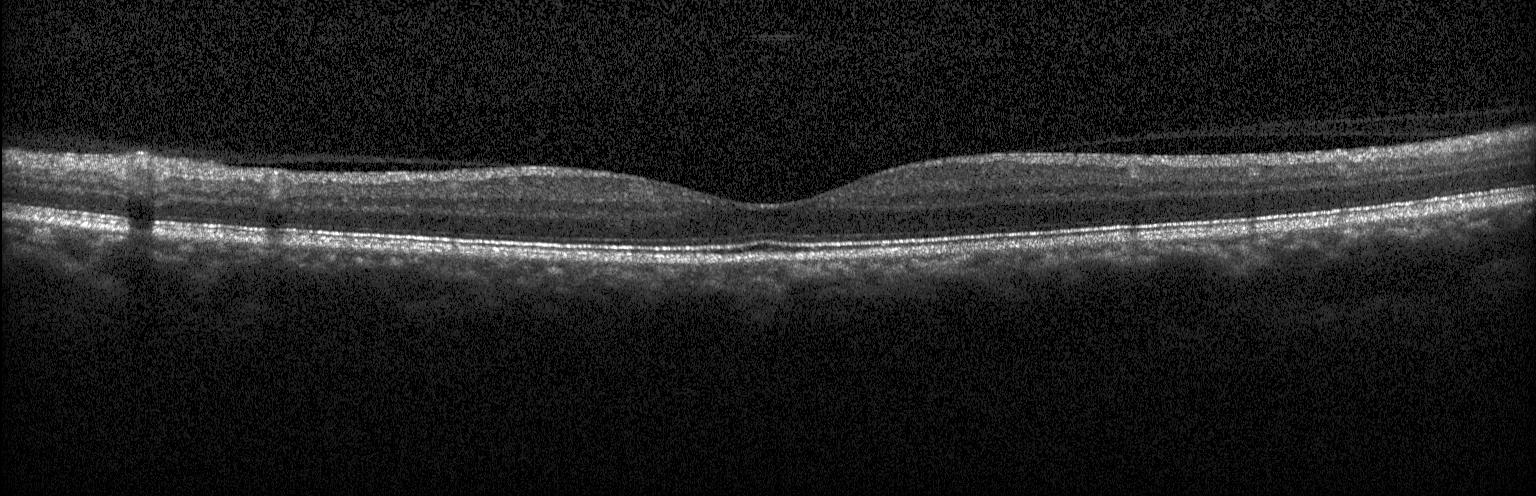
Impression: no choroidal neovascularization, diabetic macular edema, or drusen.